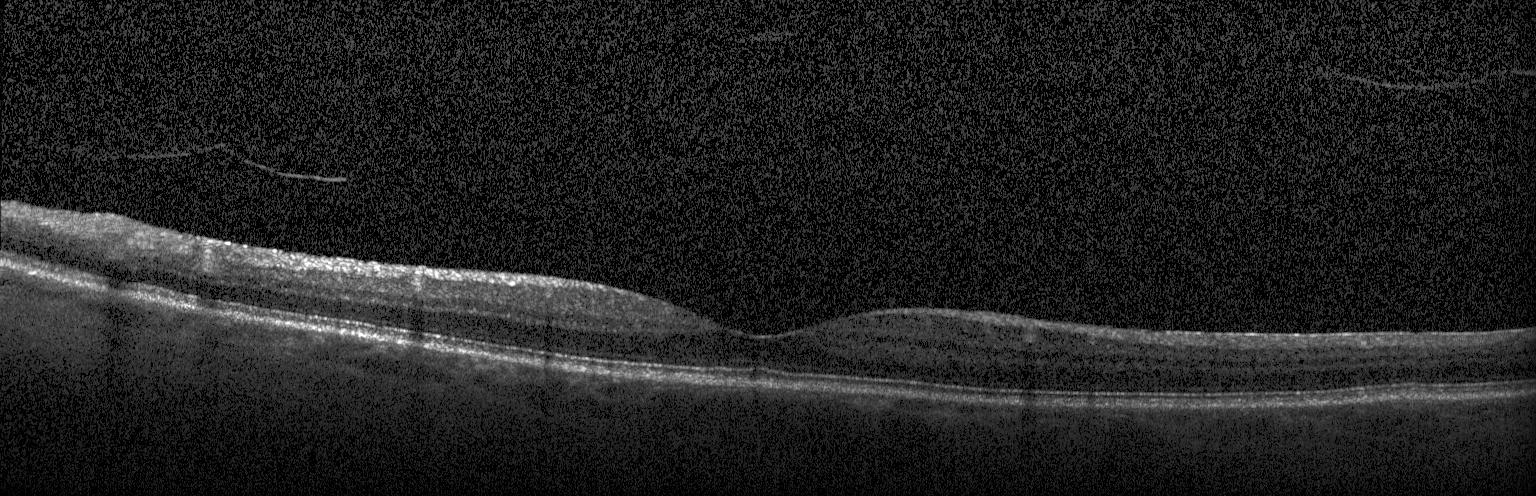 Spectral-domain OCT; OCT line scan; acquired on a Heidelberg Spectralis
OCT finding: neither choroidal neovascularization, diabetic macular edema, nor drusen.